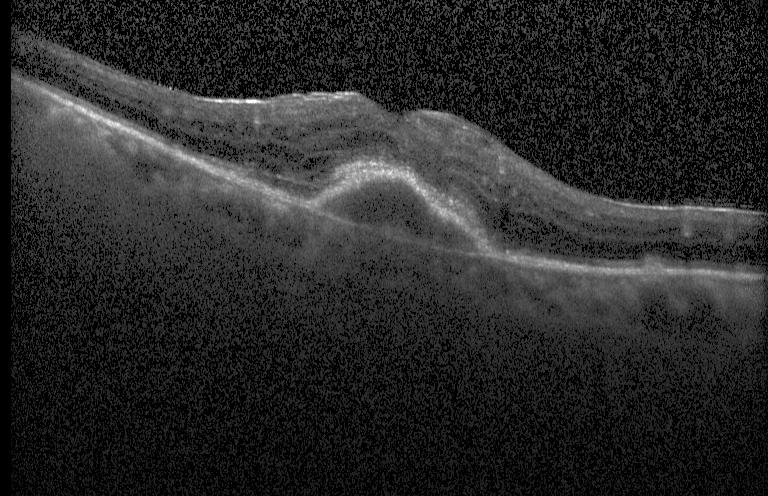 Instrument: Heidelberg Spectralis, spectral-domain OCT, optical coherence tomography scan.
Finding: choroidal neovascularization (CNV).